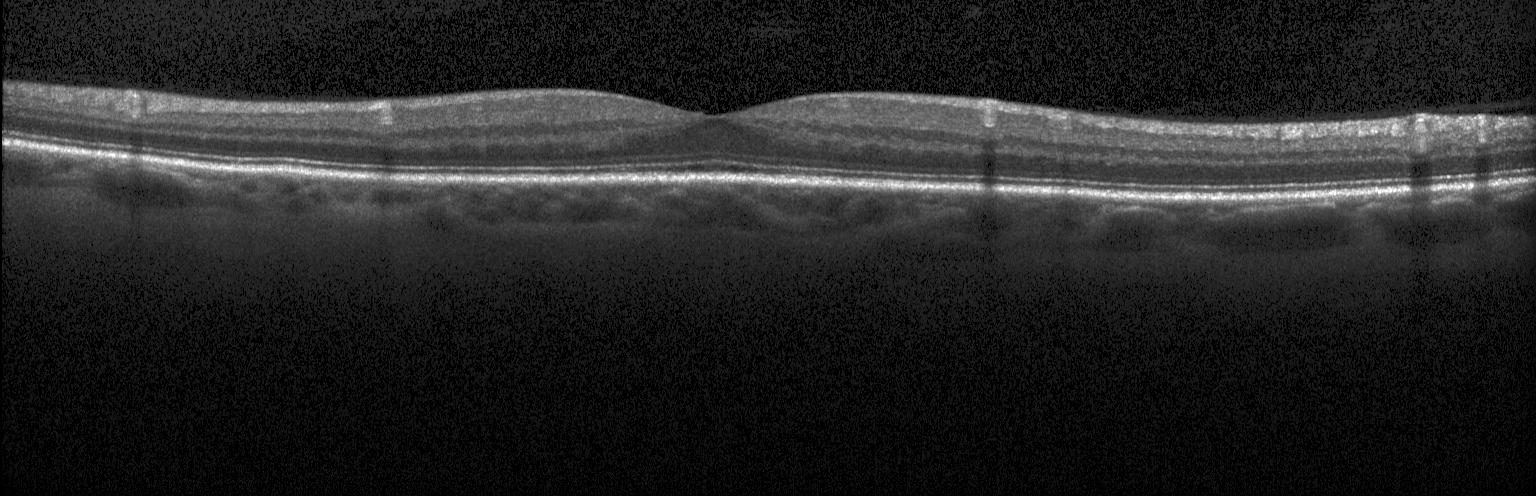 Optical coherence tomography B-scan
Dx: no CNV, no DME, and no drusen.